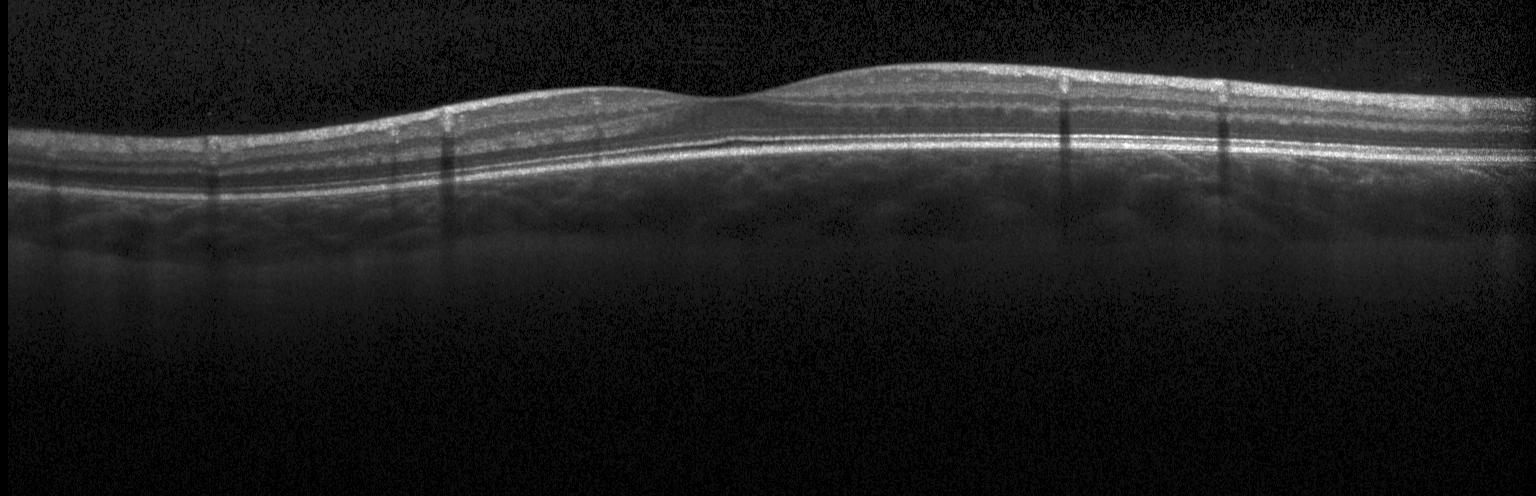

Acquired on a Heidelberg Spectralis · optical coherence tomography scan · horizontal scan through the fovea · SD-OCT.
Finding: neither choroidal neovascularization, diabetic macular edema, nor drusen.